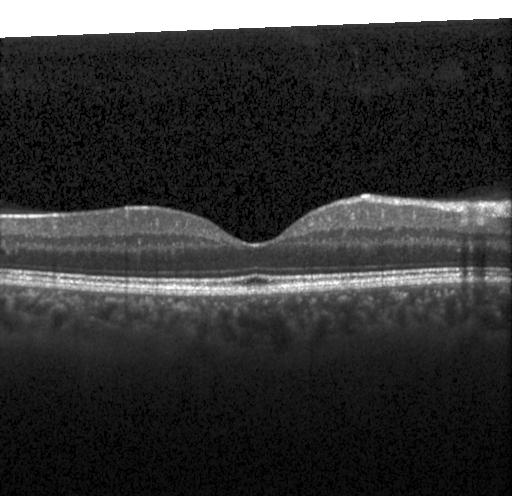

Finding: no evidence of choroidal neovascularization, diabetic macular edema, or drusen.